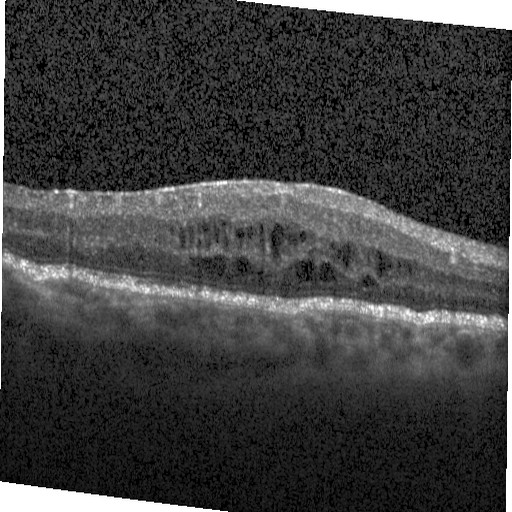

Dx: diabetic macular edema (DME).